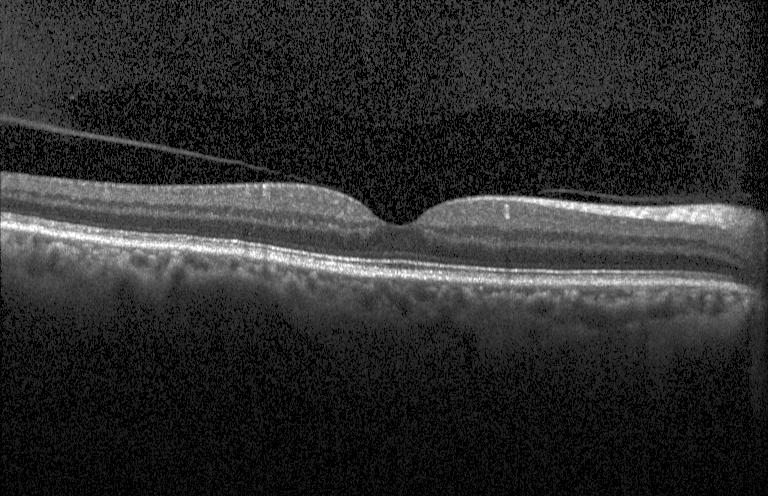

Acquired on a Heidelberg Spectralis; optical coherence tomography B-scan.
Neither choroidal neovascularization, diabetic macular edema, nor drusen.